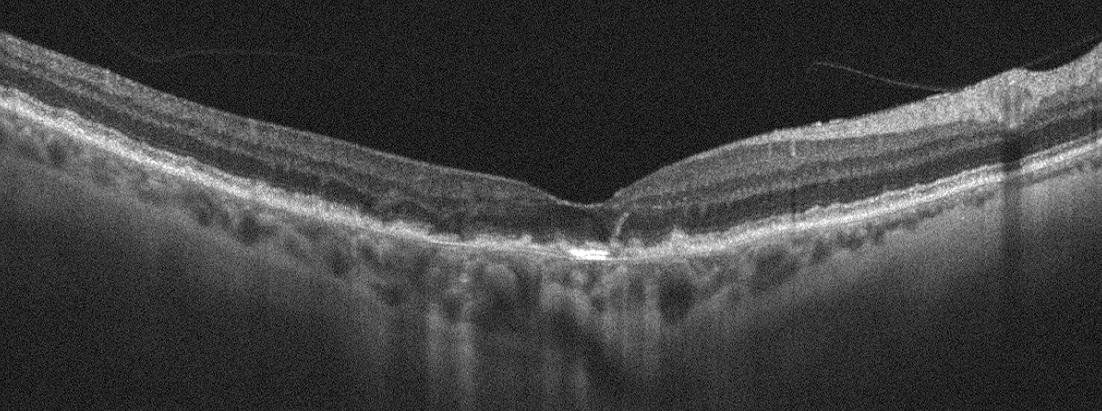 Retinal OCT cross-section; through the macula.
Finding: age-related macular degeneration.